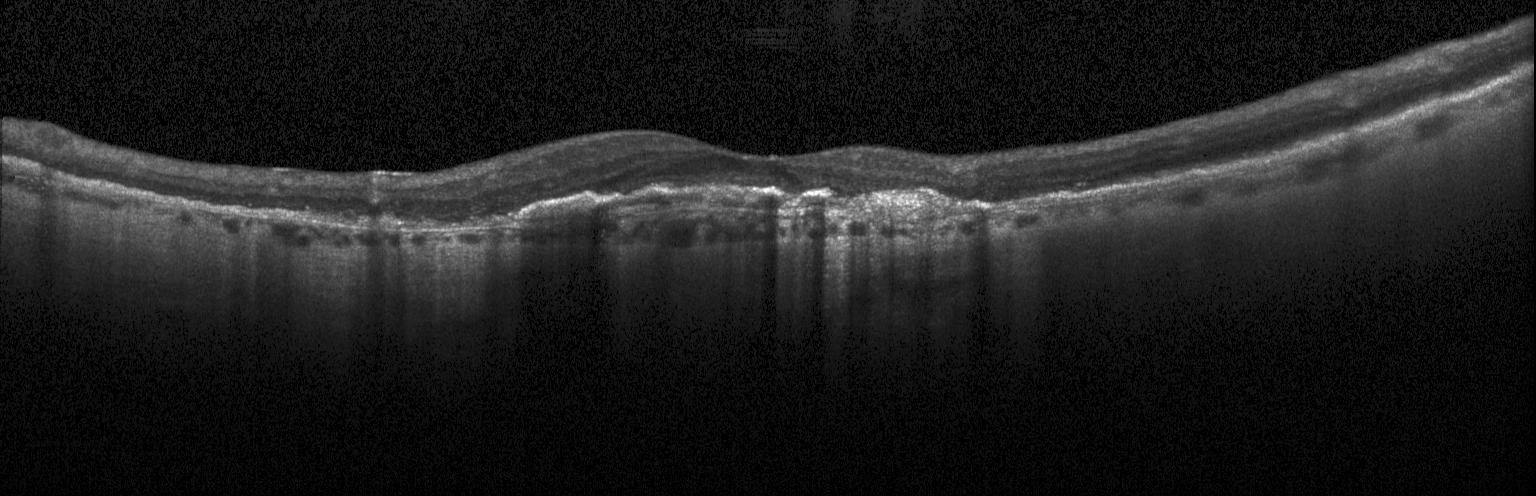

OCT B-scan — A choroidal neovascular membrane.